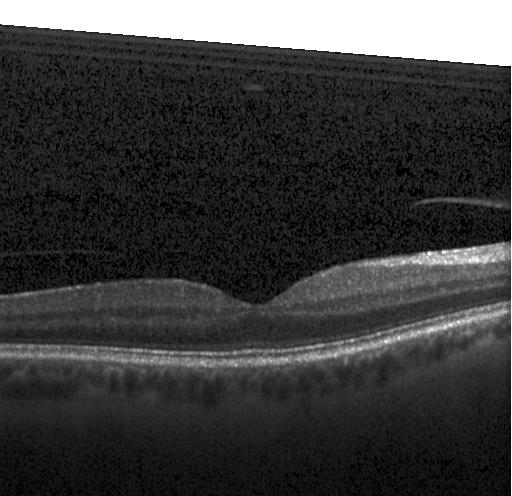

Optical coherence tomography B-scan — No CNV, DME, or drusen.